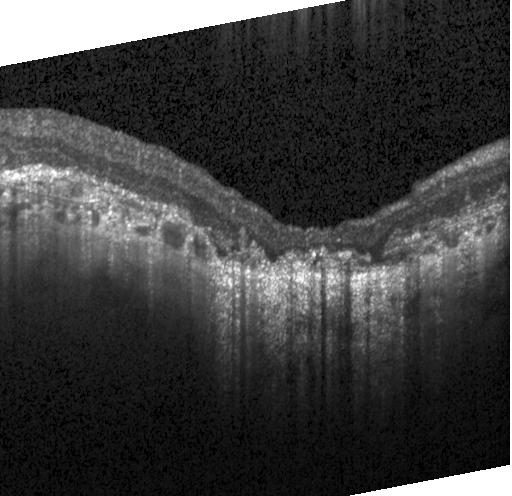
Retinal OCT B-scan — Assessment: a choroidal neovascular membrane.